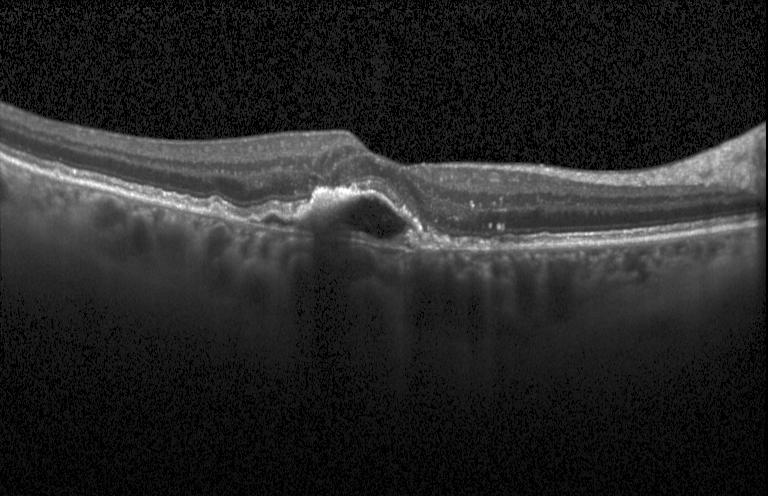 Optical coherence tomography B-scan. Diagnosis: a choroidal neovascular membrane.